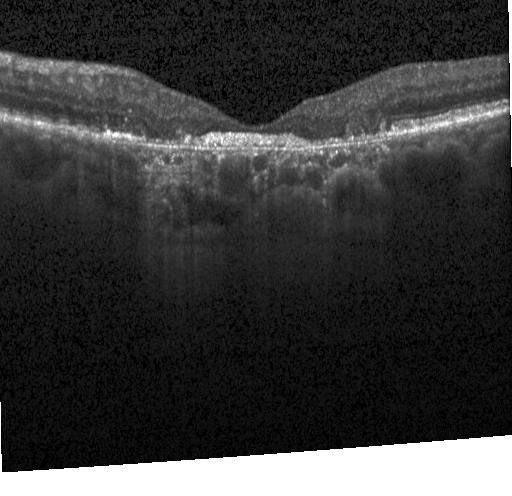 Optical coherence tomography B-scan. Dx: a choroidal neovascular membrane.